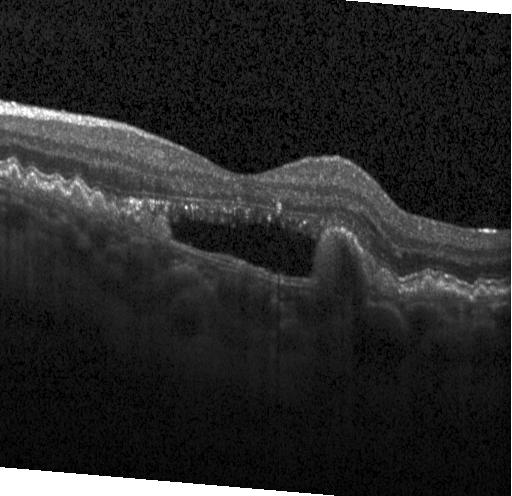

Retinal OCT B-scan; SD-OCT; centered on the fovea; acquired on a Heidelberg Spectralis — Diagnosis: a choroidal neovascular membrane.